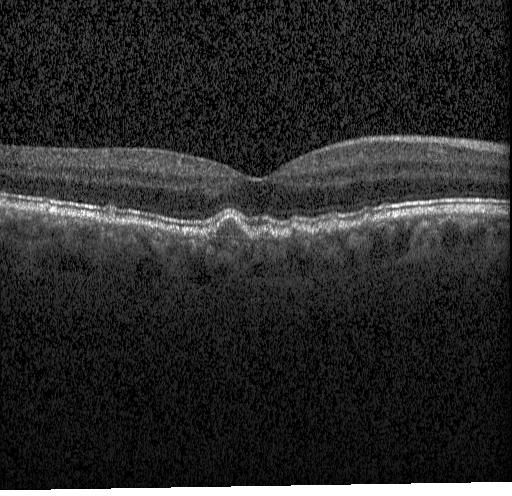 Finding: multiple drusen.